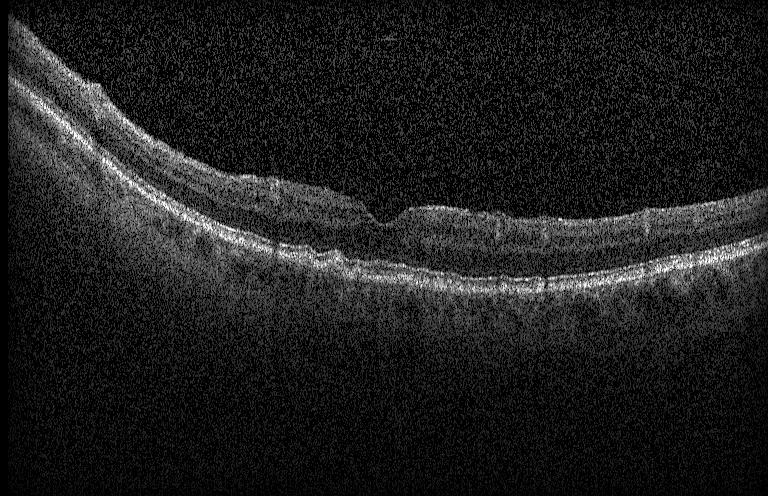
Through the macula, retinal OCT B-scan
Dx: drusen.